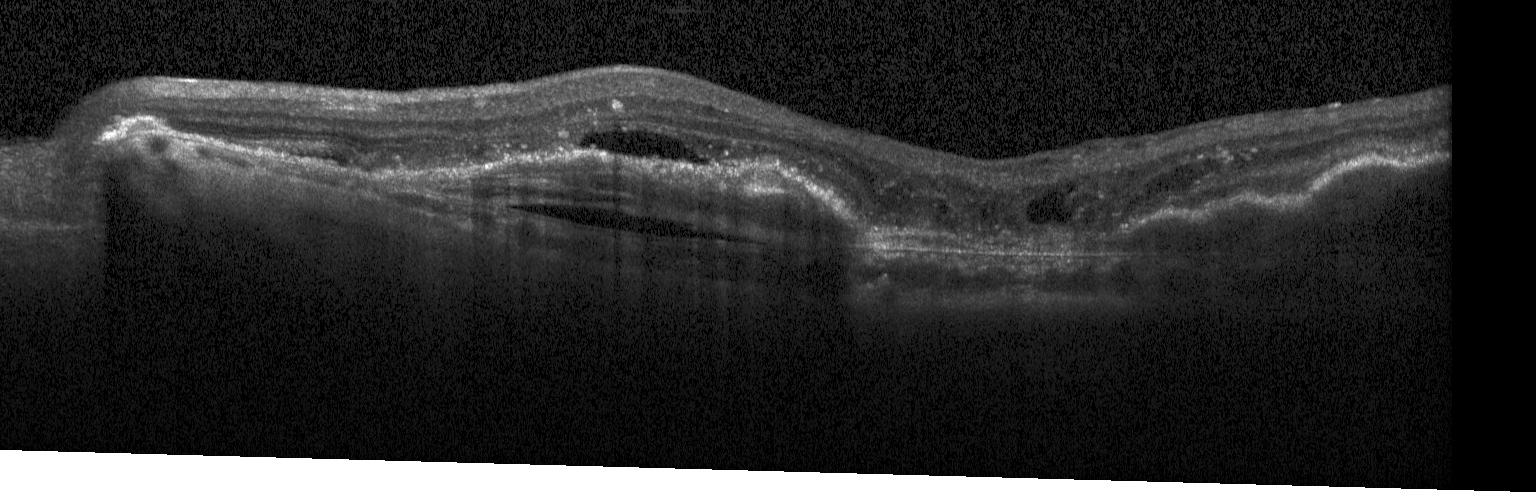
Macular OCT demonstrating choroidal neovascularization.